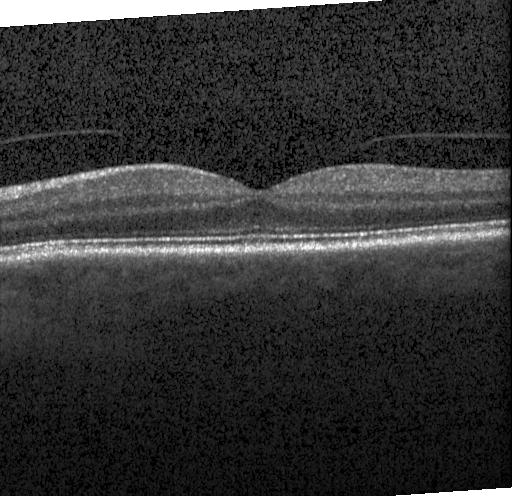
Heidelberg Spectralis OCT system. Optical coherence tomography scan. Macular scan — OCT finding: neither choroidal neovascularization, diabetic macular edema, nor drusen.